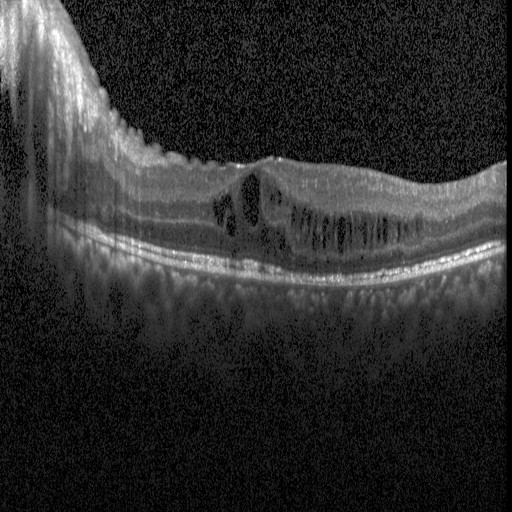

Dx: DME.